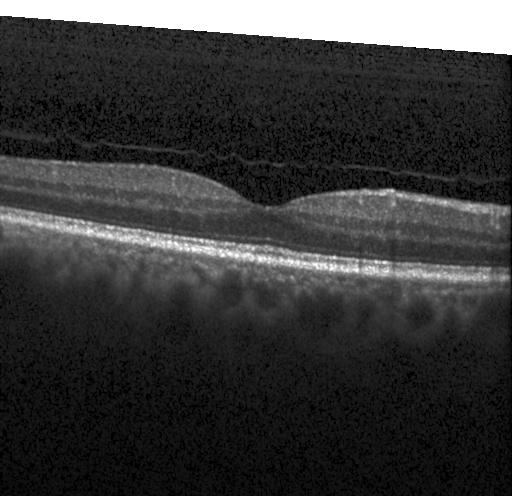
OCT B-scan.
Impression: neither choroidal neovascularization, diabetic macular edema, nor drusen.